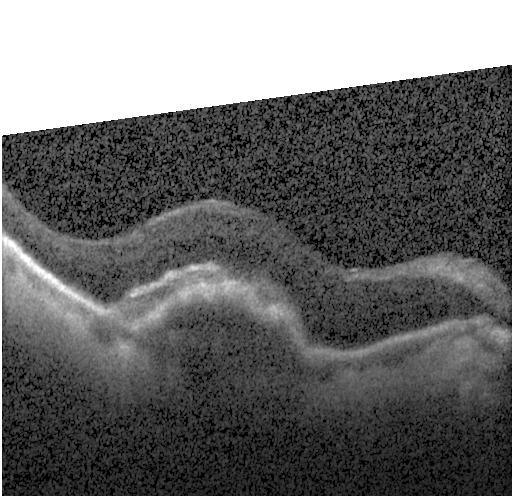
OCT B-scan.
Dx: choroidal neovascularization (CNV).